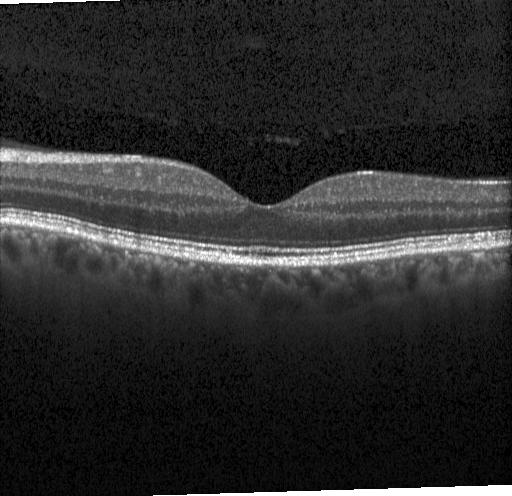 Spectral-domain optical coherence tomography; Heidelberg Spectralis; optical coherence tomography B-scan; horizontal scan through the fovea. Diagnosis: neither choroidal neovascularization, diabetic macular edema, nor drusen.